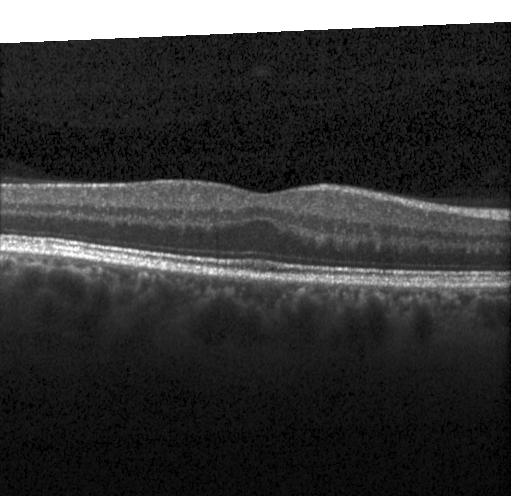
No choroidal neovascularization, no diabetic macular edema, and no drusen.